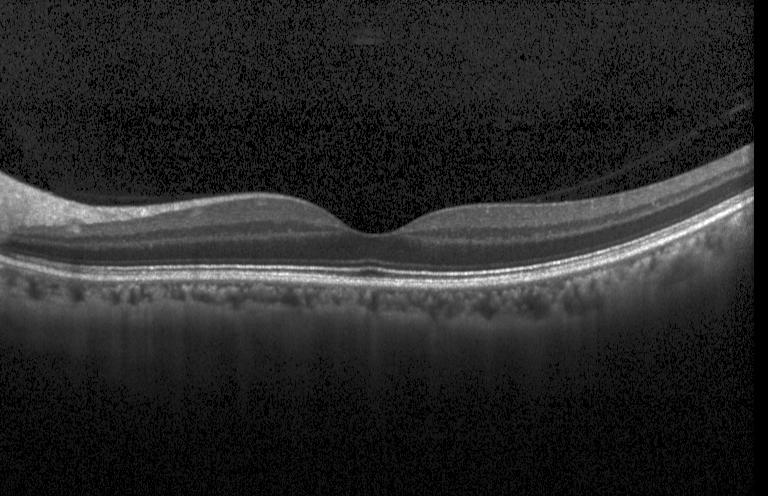

Spectral-domain OCT B-scan: no choroidal neovascularization, no diabetic macular edema, and no drusen.